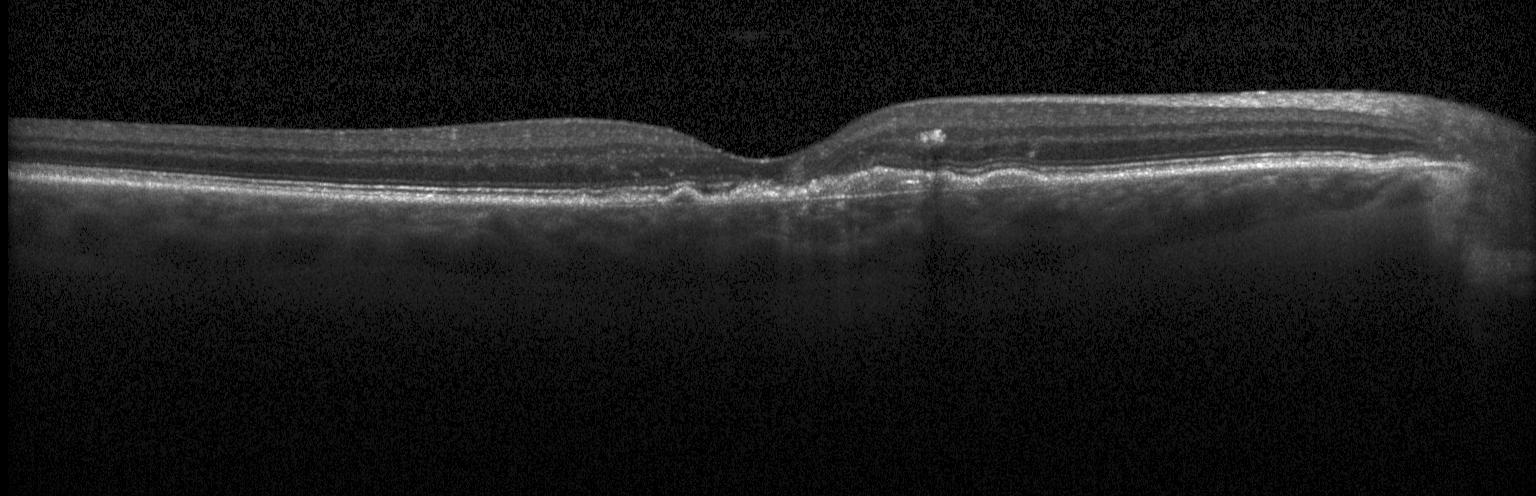
OCT B-scan, Heidelberg Spectralis OCT system, horizontal scan through the fovea.
Impression: choroidal neovascularization.